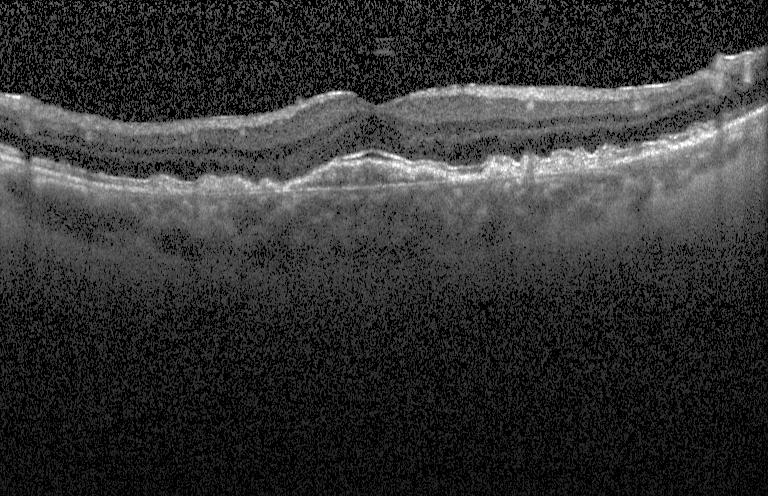
Impression: CNV.